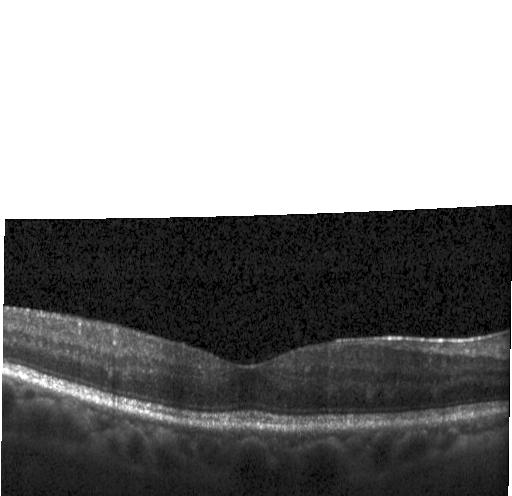

OCT B-scan. Dx: neither CNV, DME, nor drusen.